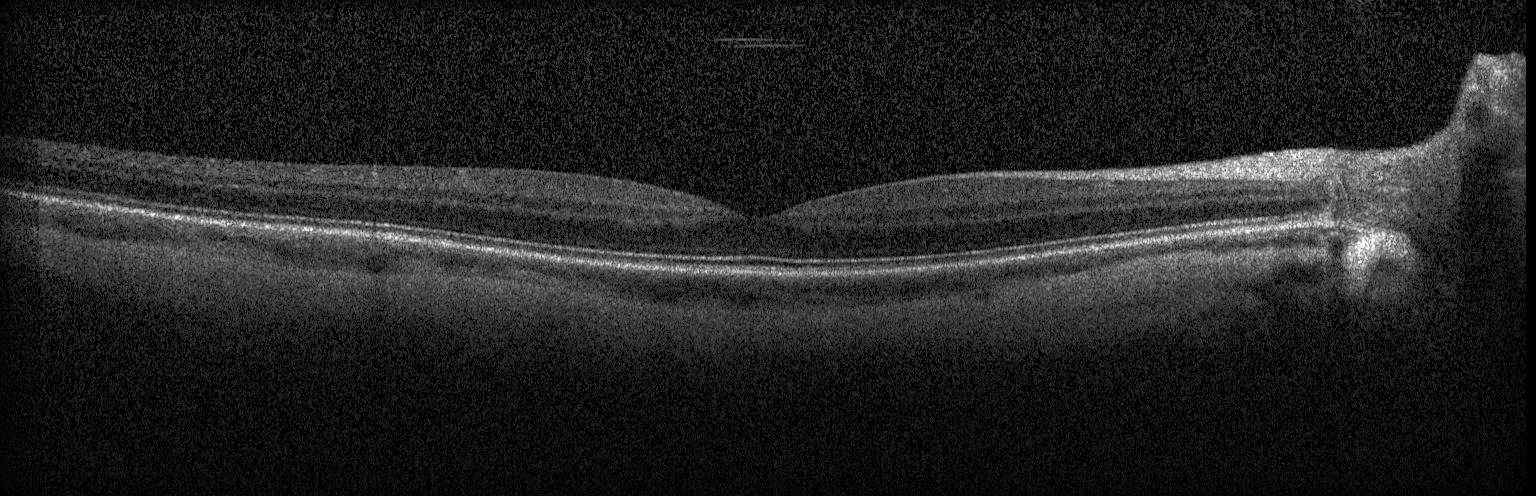
Optical coherence tomography scan — Macular OCT: neither choroidal neovascularization, diabetic macular edema, nor drusen.